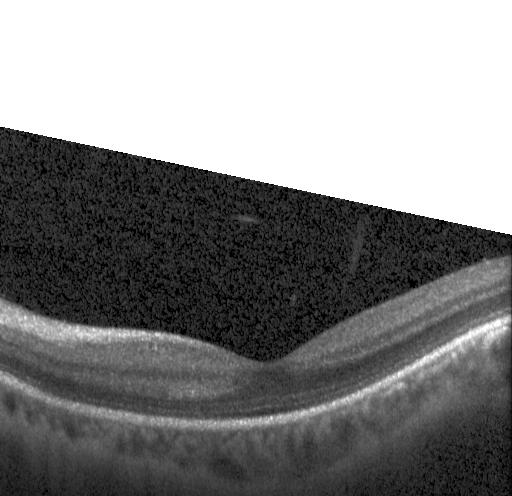 Macular OCT: no evidence of CNV, DME, or drusen.